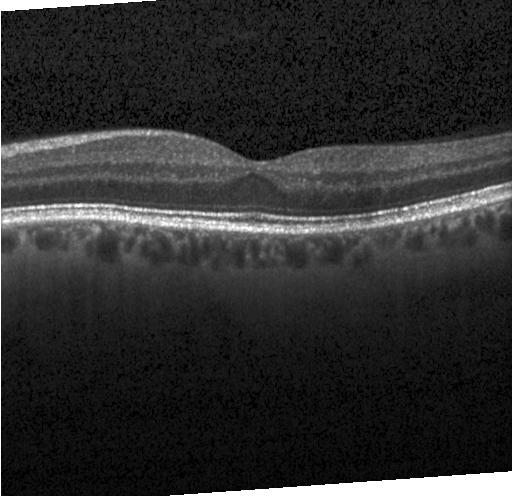 OCT B-scan showing no choroidal neovascularization, no diabetic macular edema, and no drusen.